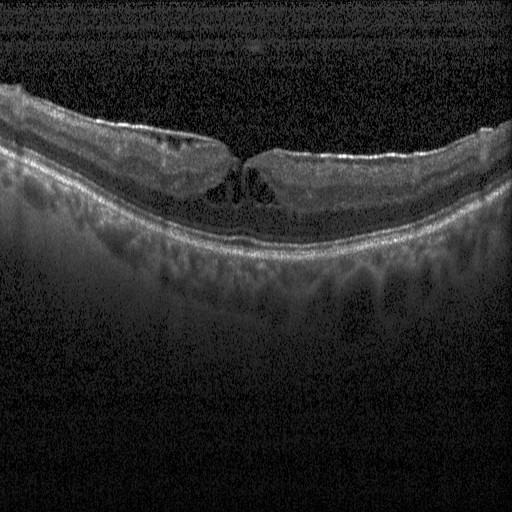 Spectral-domain optical coherence tomography, OCT line scan — Finding: diabetic macular edema.